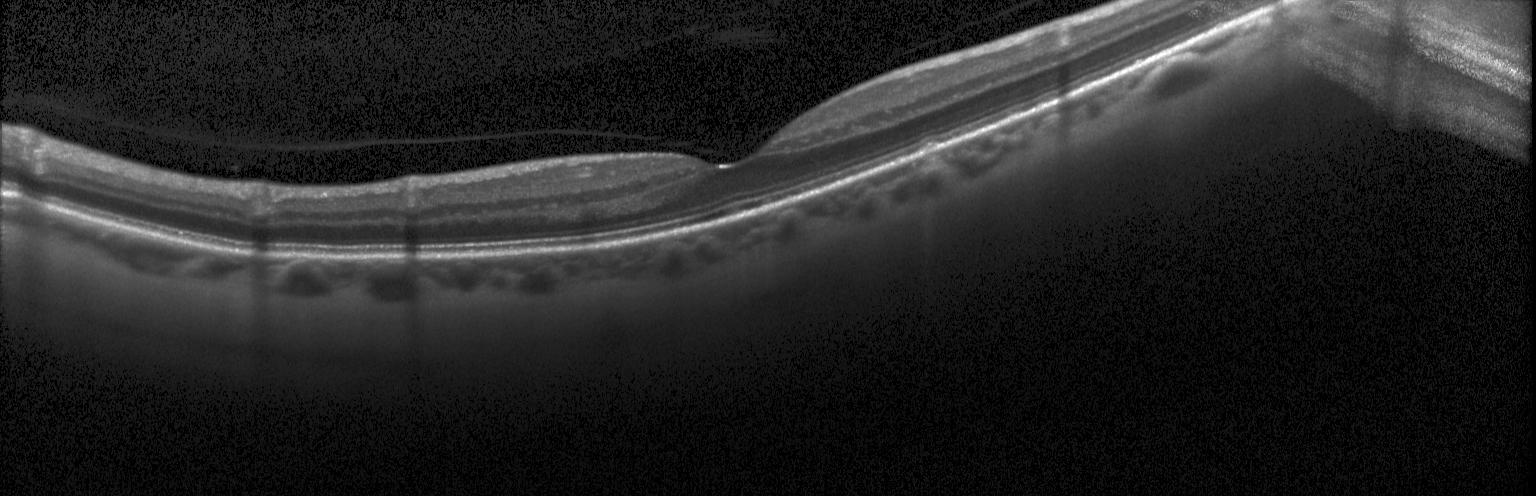
Centered on the fovea · OCT line scan · spectral-domain OCT
This B-scan demonstrates no CNV, no DME, and no drusen.